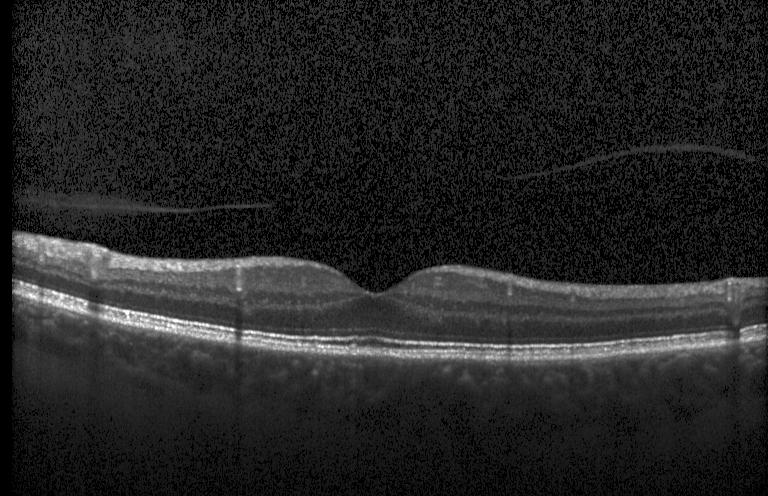

Impression: no CNV, no DME, and no drusen.